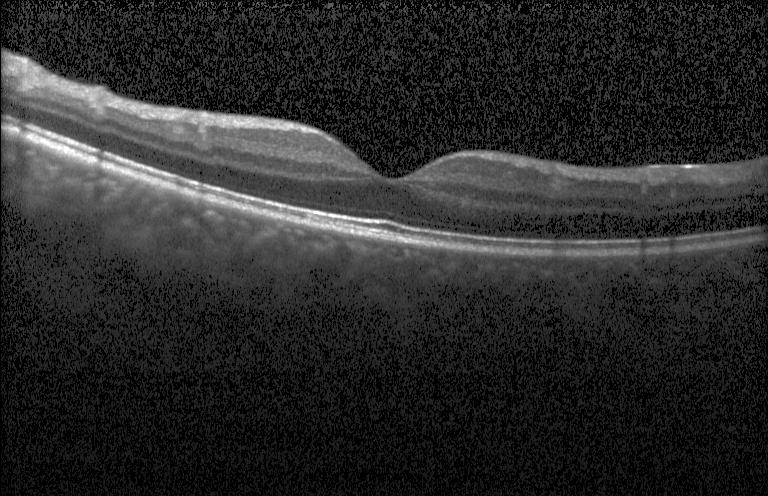
Horizontal scan through the fovea, OCT B-scan.
Diagnosis: neither CNV, DME, nor drusen.